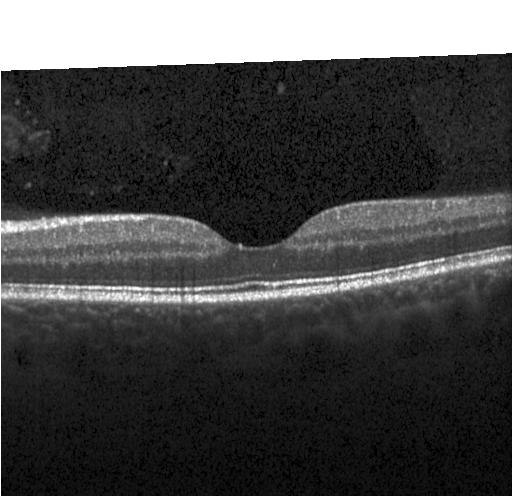 Retinal OCT cross-section. Neither choroidal neovascularization, diabetic macular edema, nor drusen.